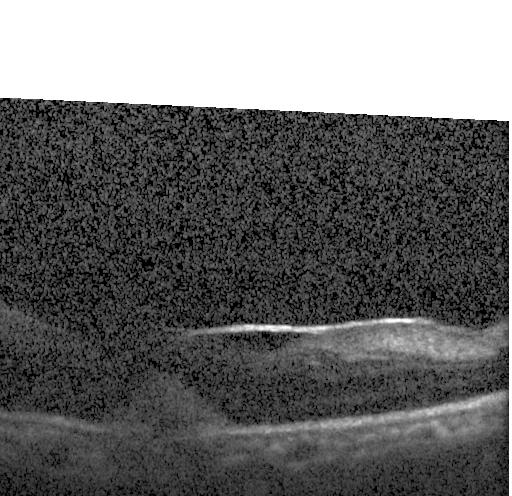
OCT line scan, acquired on a Heidelberg Spectralis, spectral-domain OCT, fovea-centered.
The scan shows choroidal neovascularization (CNV).